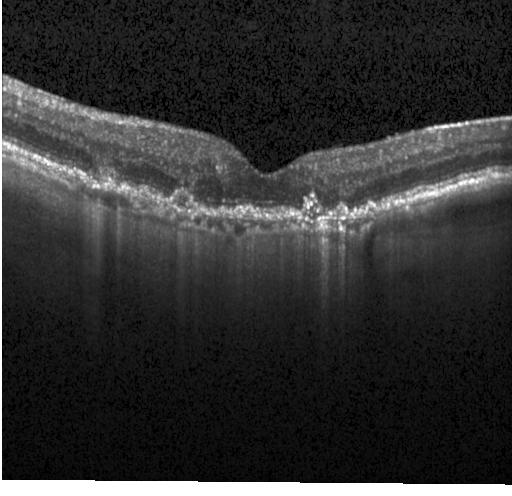

The scan shows a choroidal neovascular membrane.